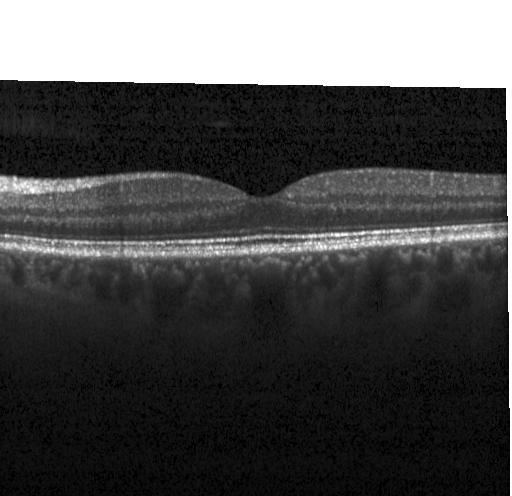
Spectral-domain optical coherence tomography. Horizontal scan through the fovea. Optical coherence tomography scan. Heidelberg Spectralis.
The scan shows neither choroidal neovascularization, diabetic macular edema, nor drusen.